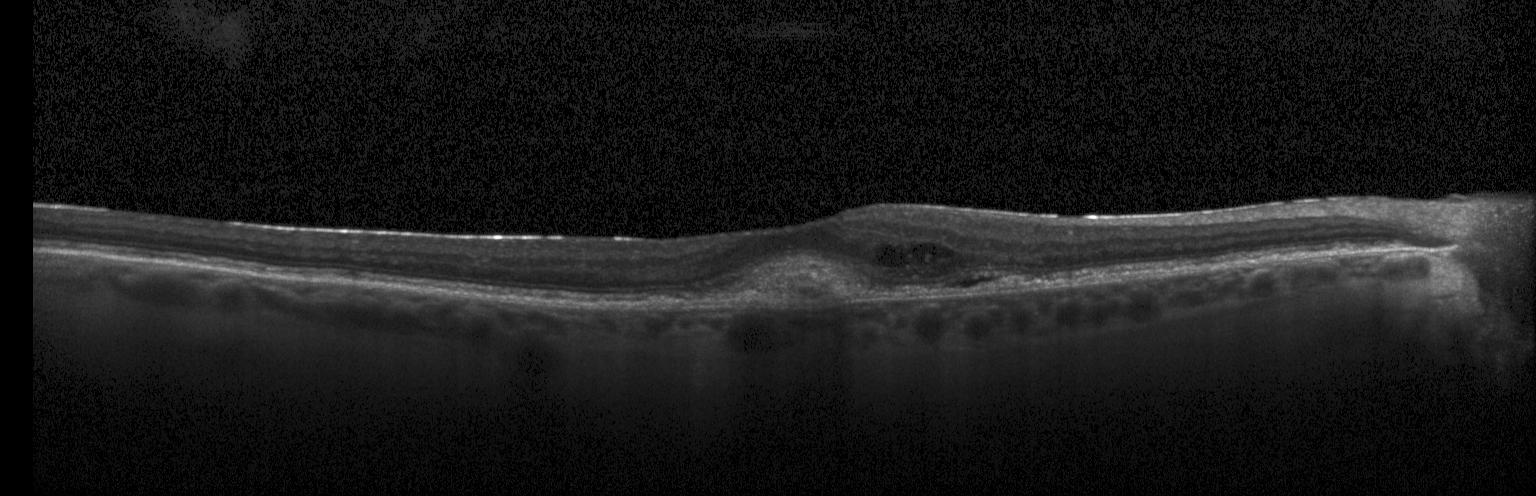

Assessment: CNV.